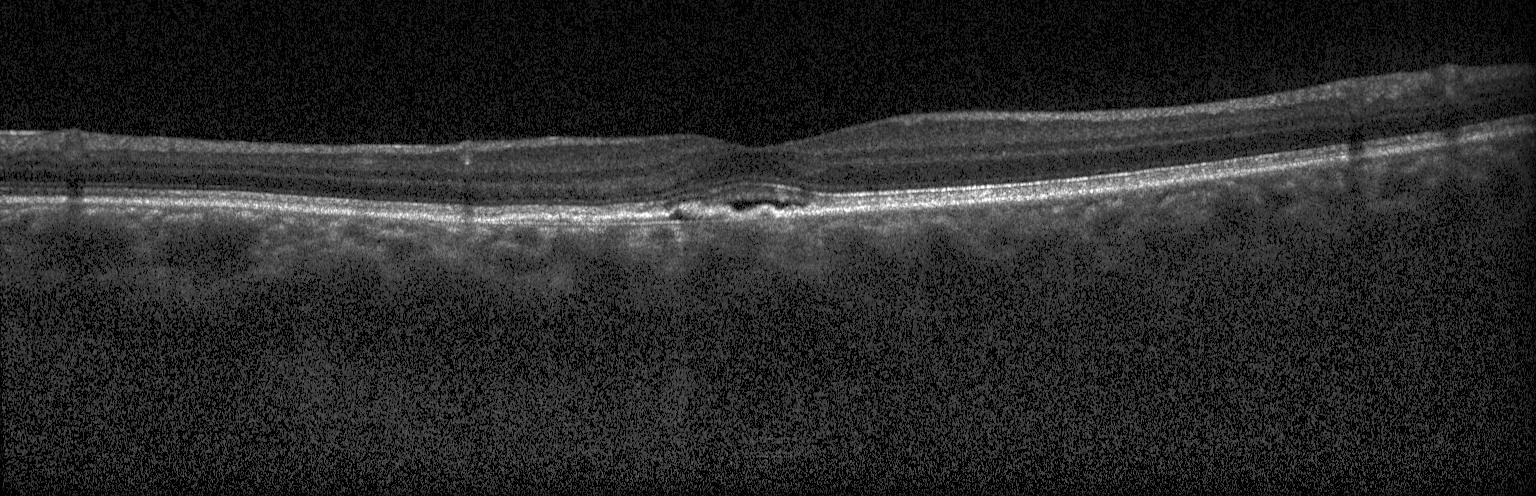

OCT line scan, Heidelberg Spectralis, SD-OCT
OCT finding: choroidal neovascularization (CNV).